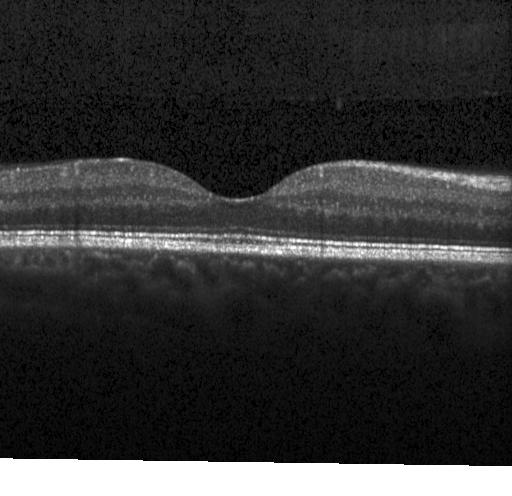 No choroidal neovascularization, no diabetic macular edema, and no drusen.